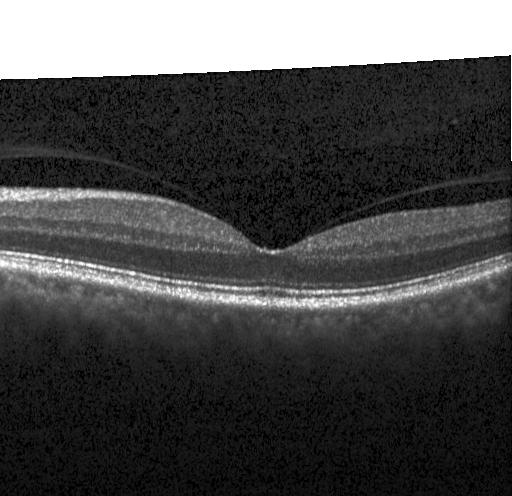
Spectral-domain optical coherence tomography · retinal OCT cross-section — Macular OCT: no evidence of CNV, DME, or drusen.